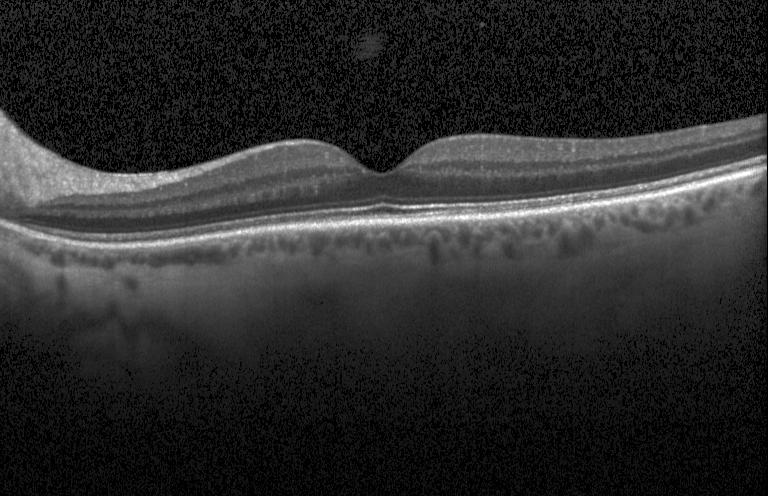 OCT B-scan. Diagnosis: no evidence of CNV, DME, or drusen.